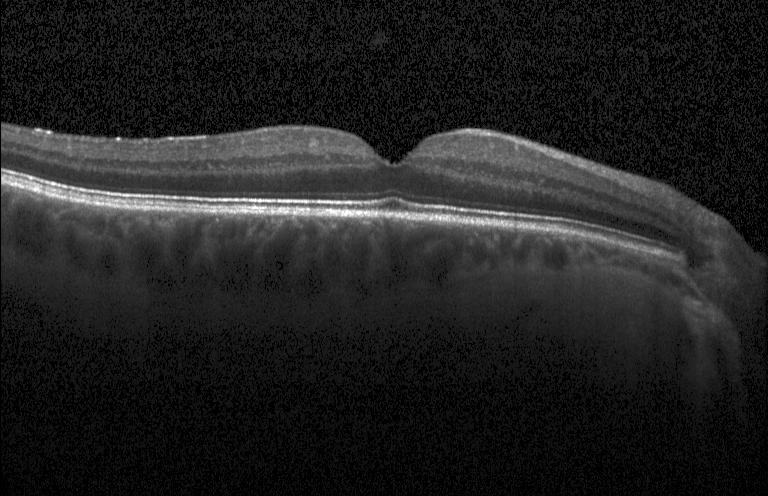 Macular OCT: no CNV, DME, or drusen.